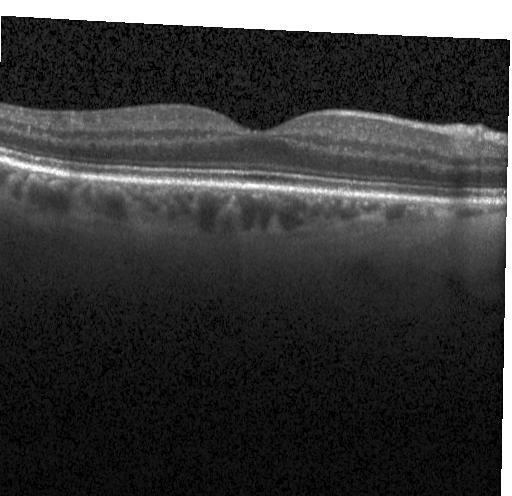 Macular OCT demonstrating no choroidal neovascularization, no diabetic macular edema, and no drusen.